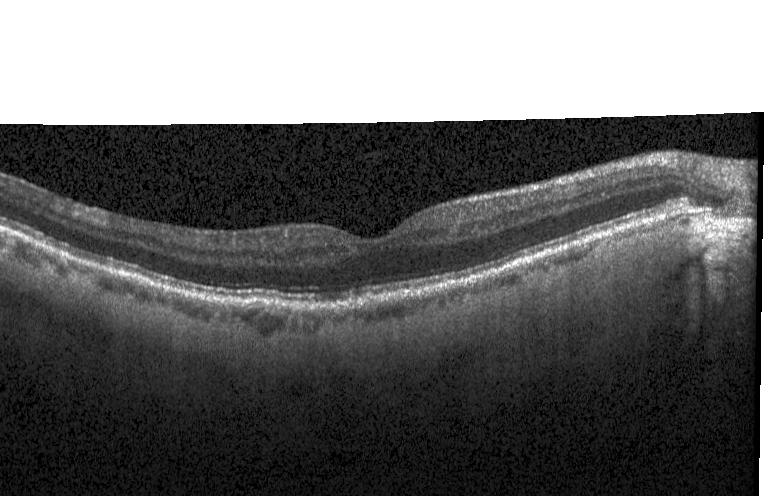
Through the macula; OCT B-scan
The scan shows no choroidal neovascularization, diabetic macular edema, or drusen.